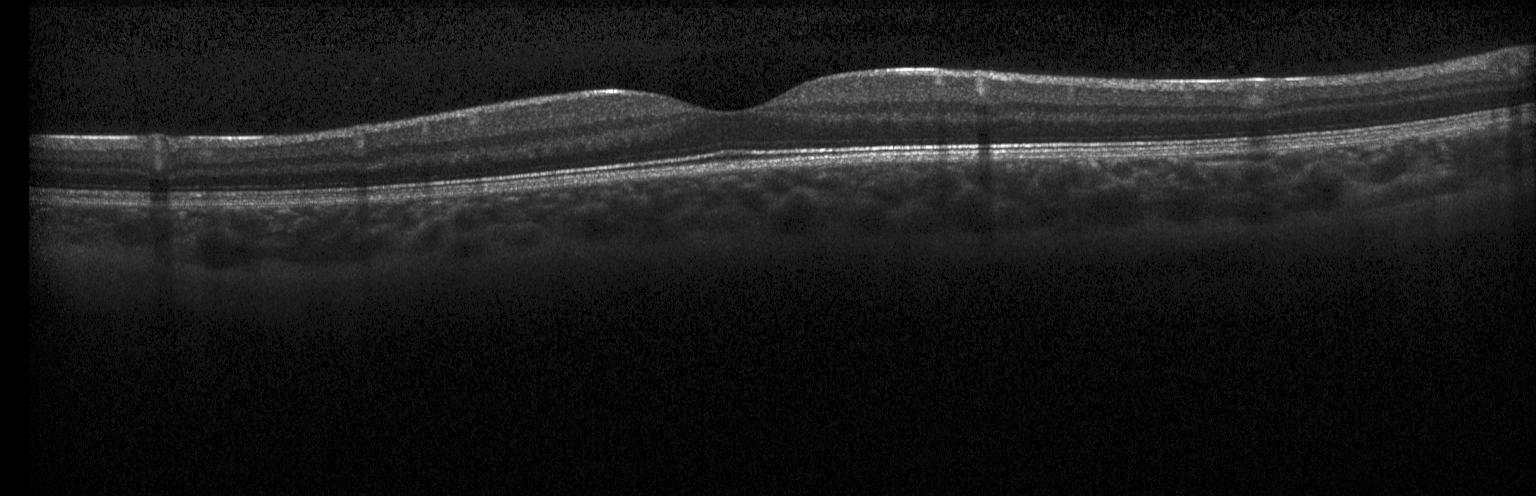

Finding: no choroidal neovascularization, diabetic macular edema, or drusen.